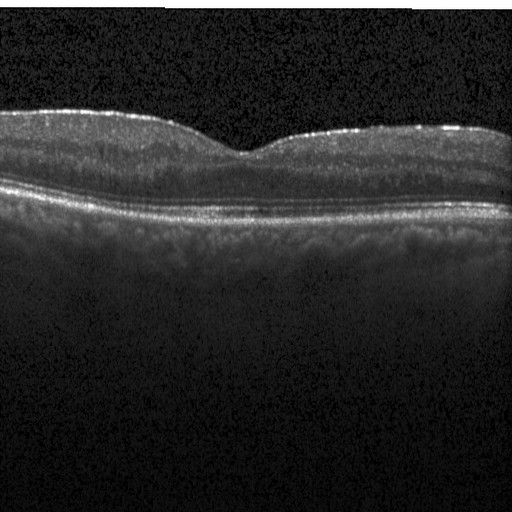
DME.